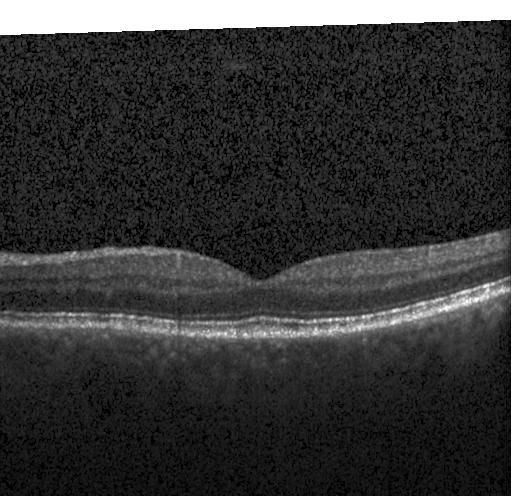

Optical coherence tomography B-scan; spectral-domain optical coherence tomography; fovea-centered. Finding: no choroidal neovascularization, diabetic macular edema, or drusen.